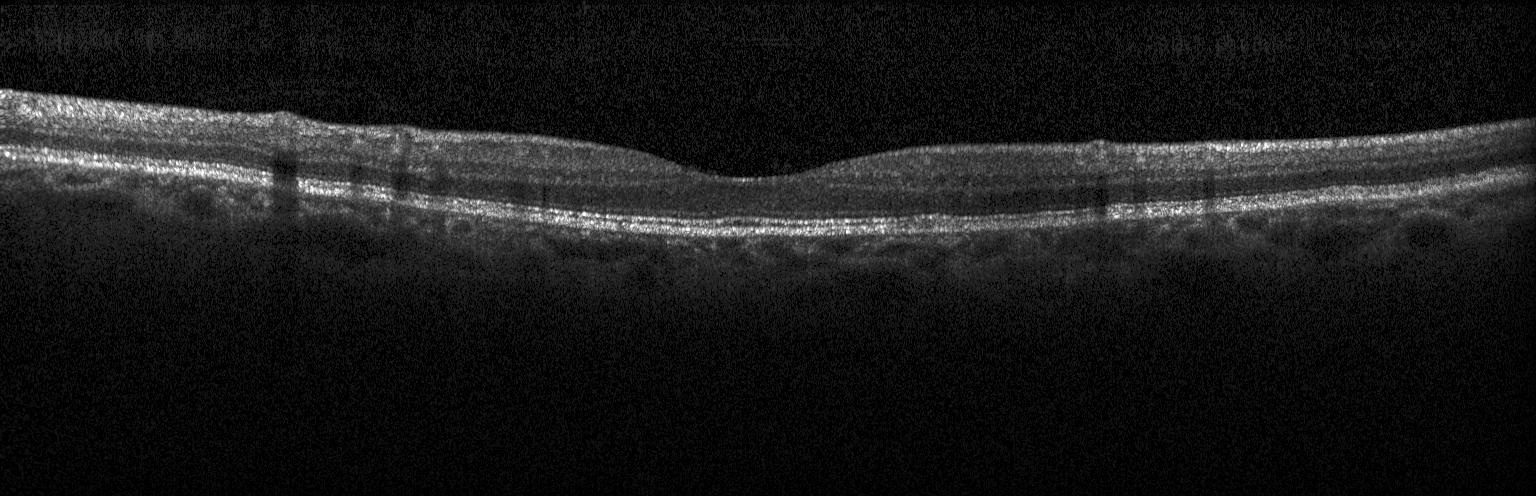 Fovea-centered. Spectral-domain OCT. Retinal OCT B-scan. Finding: no choroidal neovascularization, no diabetic macular edema, and no drusen.